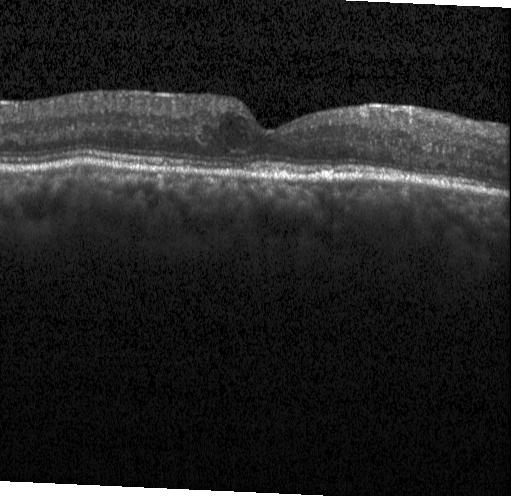 OCT B-scan
Macular OCT: DME.